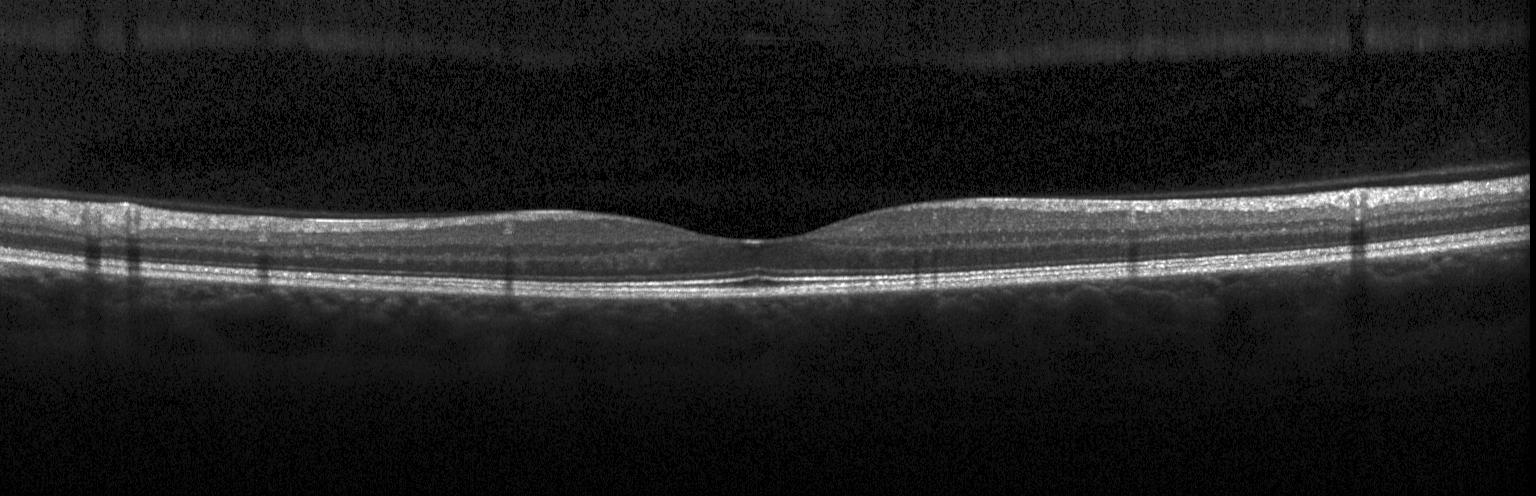

Macular OCT: neither choroidal neovascularization, diabetic macular edema, nor drusen.